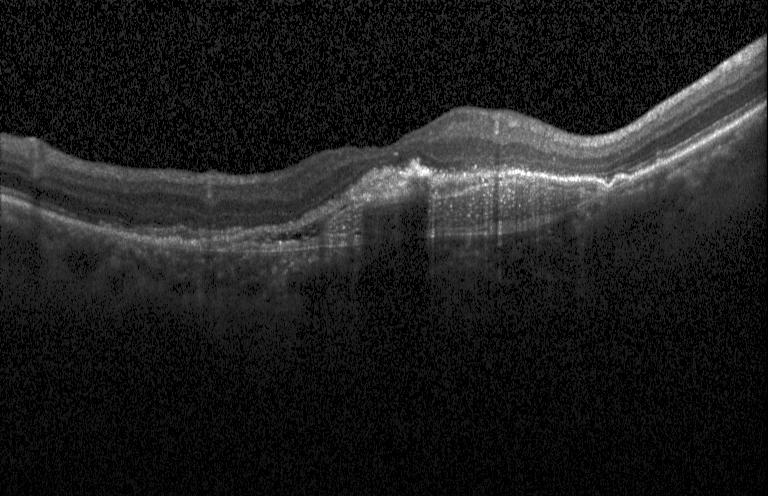 Centered on the fovea. Heidelberg Spectralis. Optical coherence tomography scan
The scan shows a choroidal neovascular membrane.